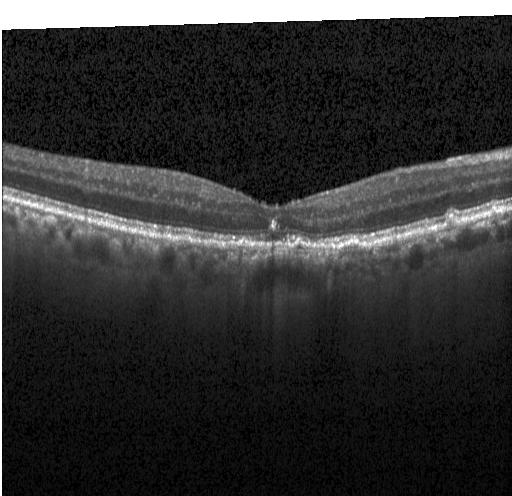

Spectral-domain OCT, retinal OCT B-scan, instrument: Heidelberg Spectralis, through the macula
Assessment: multiple drusen.